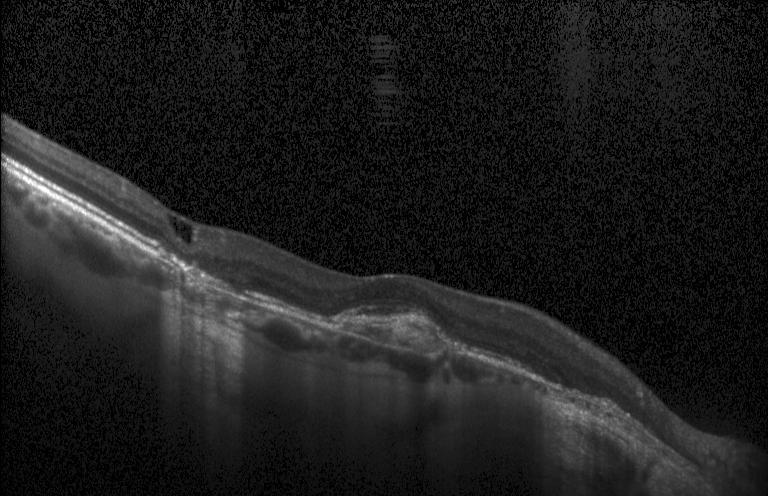 Optical coherence tomography scan
A choroidal neovascular membrane.